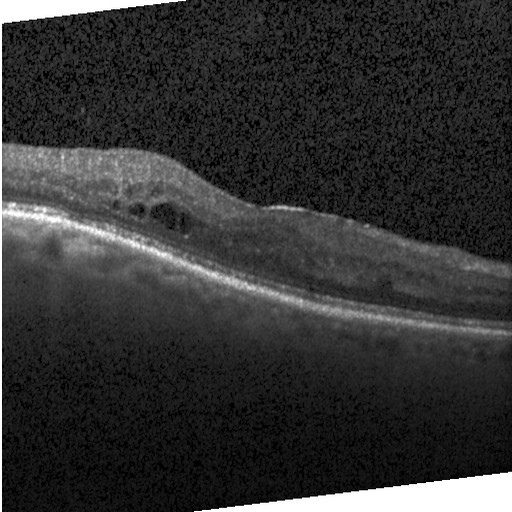
Acquired on a Heidelberg Spectralis; retinal OCT cross-section
Dx: diabetic macular edema (DME).